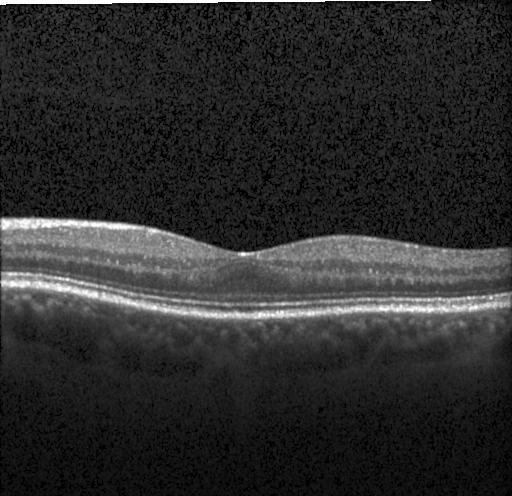 Retinal OCT B-scan · Heidelberg Spectralis. No CNV, no DME, and no drusen.